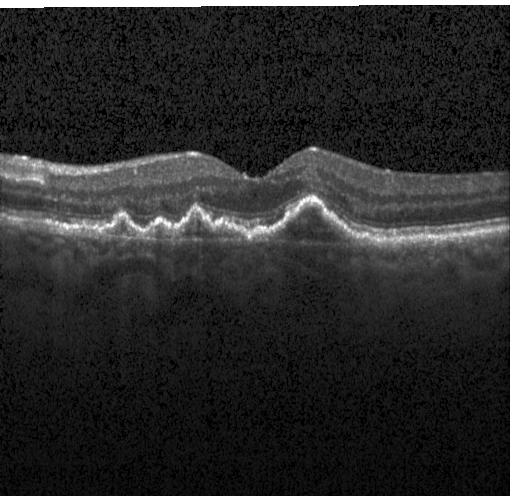 Optical coherence tomography scan — This B-scan demonstrates CNV.